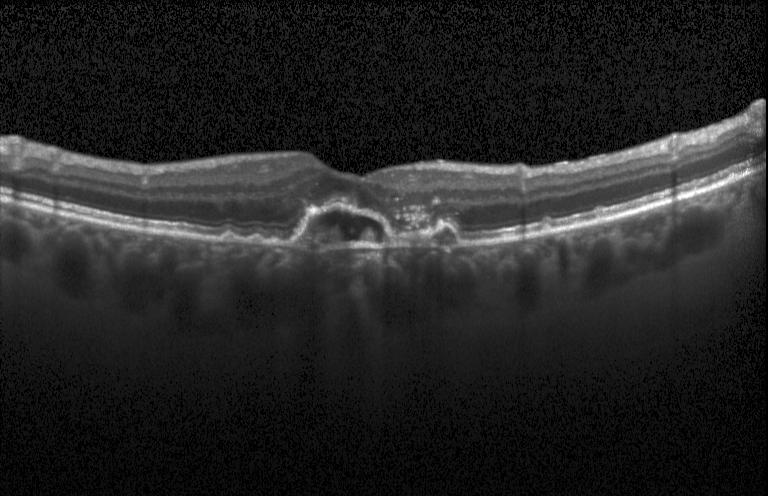 OCT finding: a choroidal neovascular membrane.